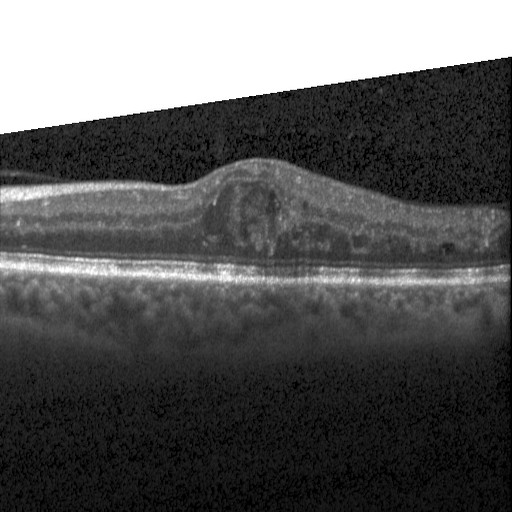

Retinal OCT B-scan — Finding: diabetic macular edema.